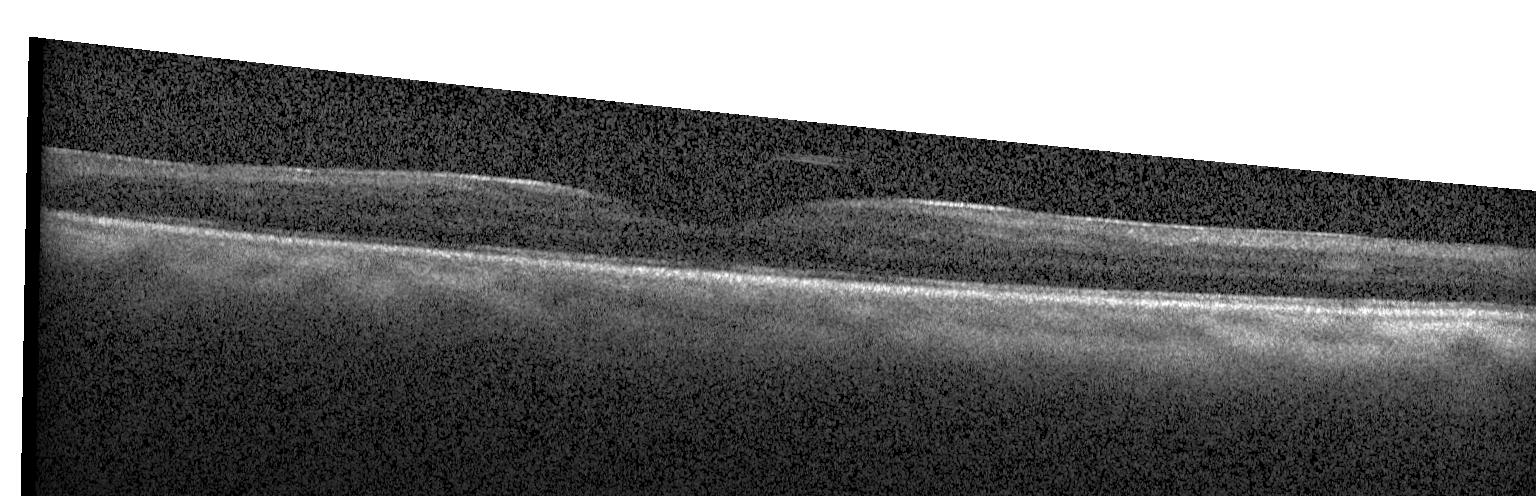 Spectral-domain OCT, OCT line scan.
Assessment: no choroidal neovascularization, diabetic macular edema, or drusen.